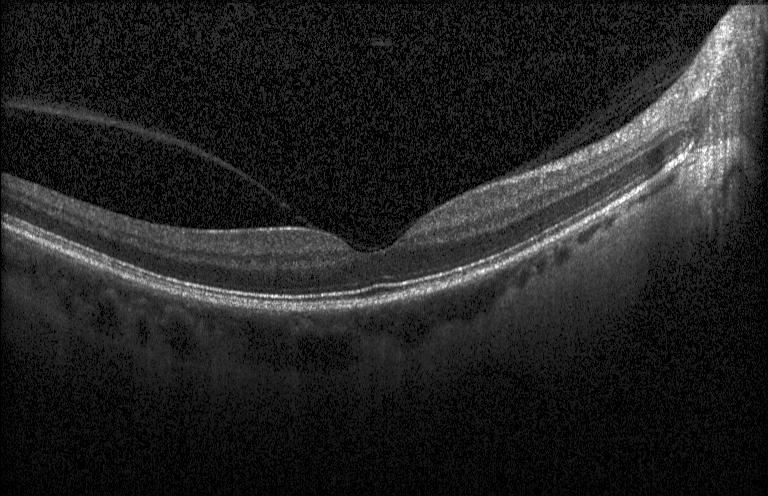
Dx: no evidence of CNV, DME, or drusen.